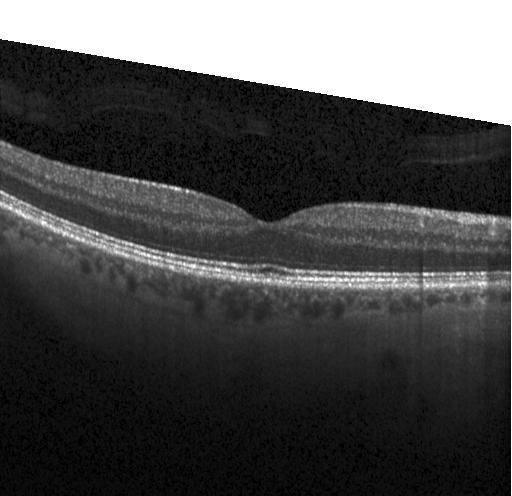

Diagnosis: neither choroidal neovascularization, diabetic macular edema, nor drusen.